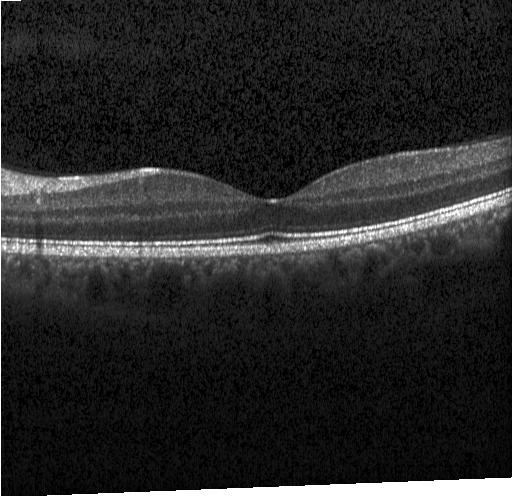

Fovea-centered · optical coherence tomography scan · instrument: Heidelberg Spectralis.
This B-scan demonstrates no choroidal neovascularization, diabetic macular edema, or drusen.